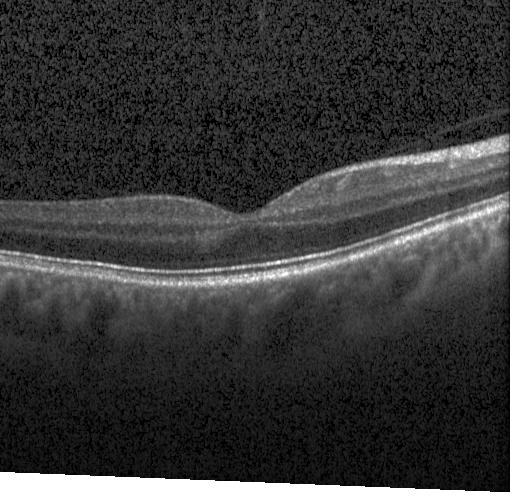 SD-OCT, through the macula, instrument: Heidelberg Spectralis, optical coherence tomography B-scan
This B-scan demonstrates no choroidal neovascularization, no diabetic macular edema, and no drusen.